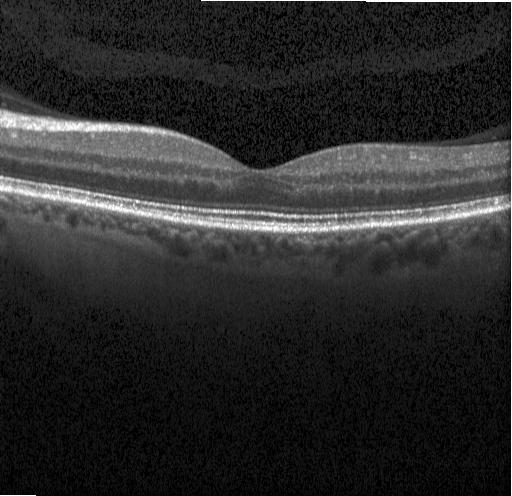
Optical coherence tomography scan; Heidelberg Spectralis OCT system.
Diagnosis: no choroidal neovascularization, diabetic macular edema, or drusen.